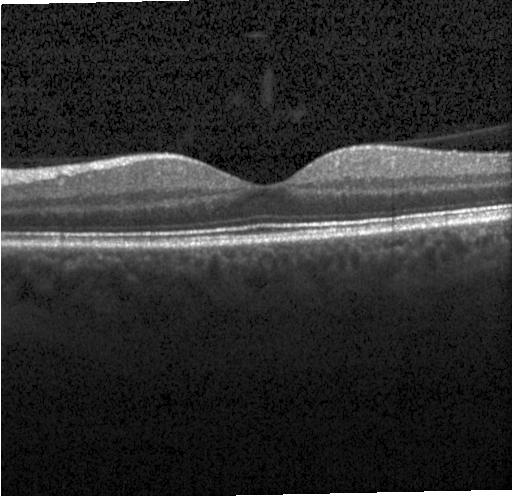

SD-OCT, OCT line scan, macular scan — Macular OCT: neither choroidal neovascularization, diabetic macular edema, nor drusen.